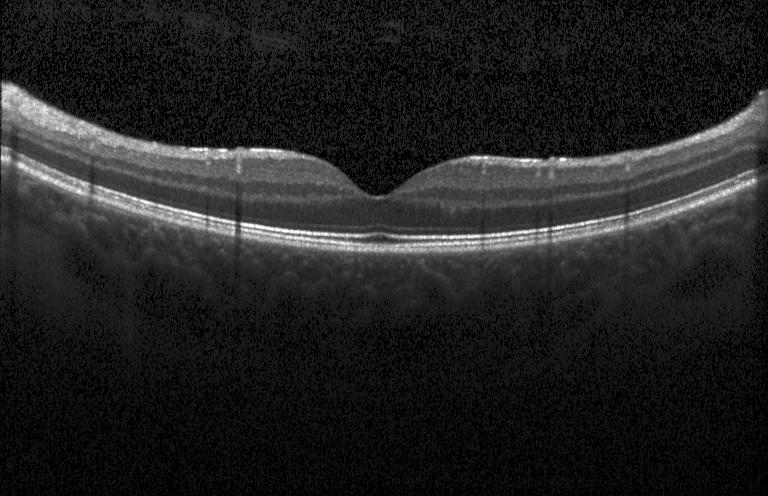 Diagnosis: no CNV, DME, or drusen.